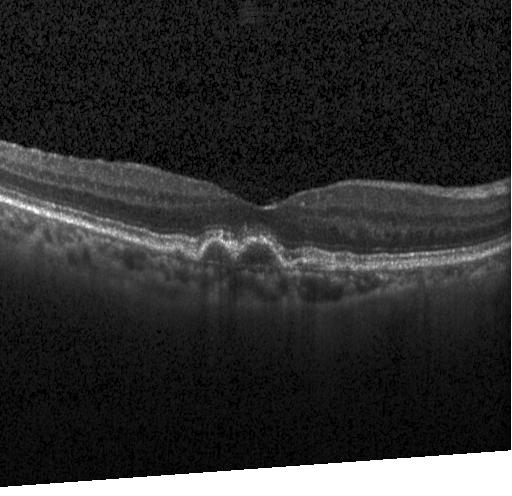

OCT B-scan showing a choroidal neovascular membrane.